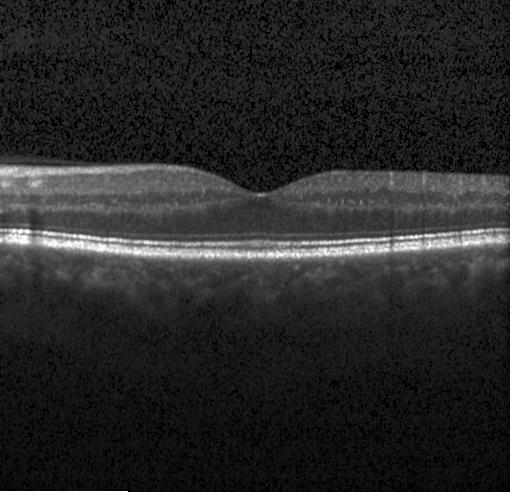
Spectral-domain OCT; horizontal scan through the fovea; optical coherence tomography scan; Heidelberg Spectralis
Diagnosis: no evidence of CNV, DME, or drusen.